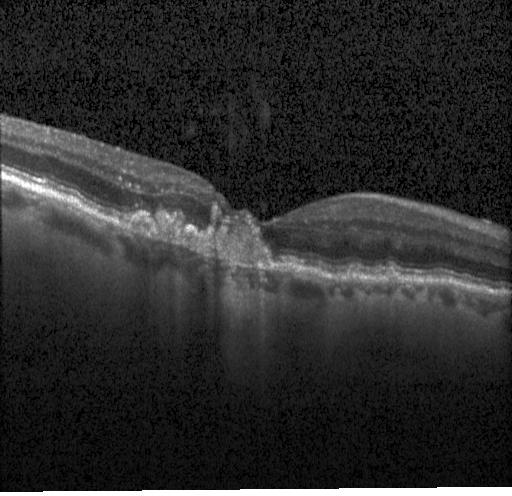

Optical coherence tomography B-scan, Heidelberg Spectralis.
Diagnosis: choroidal neovascularization.